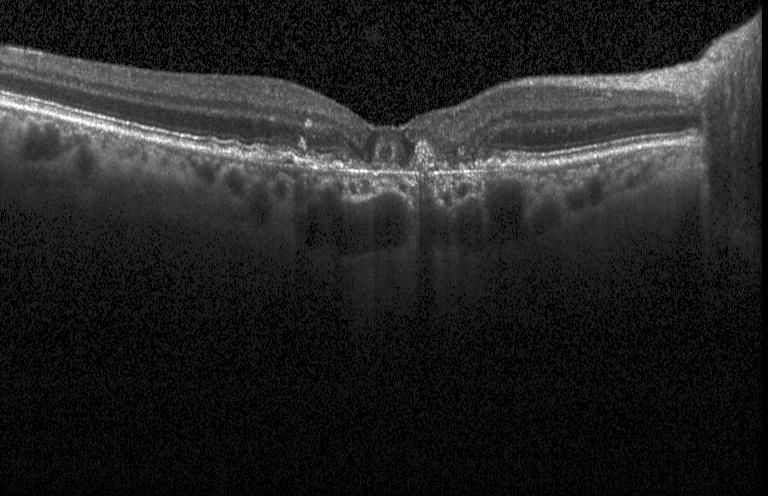
The scan shows a choroidal neovascular membrane.